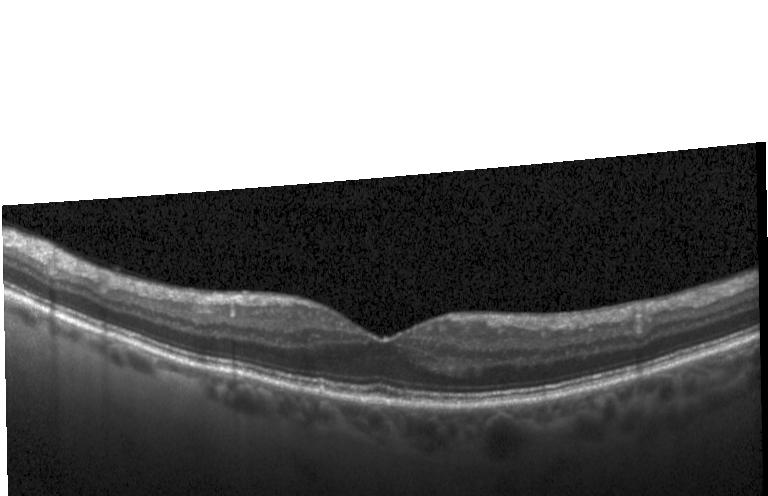 OCT scan showing no choroidal neovascularization, diabetic macular edema, or drusen.